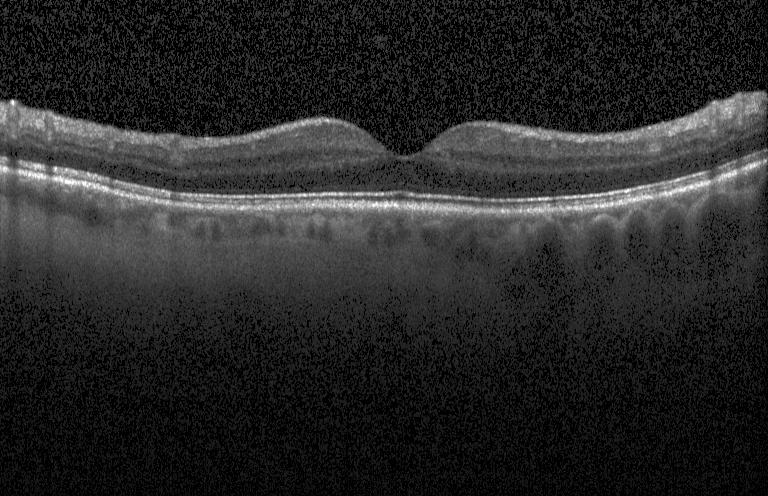
Spectral-domain optical coherence tomography · retinal OCT cross-section · horizontal scan through the fovea.
OCT finding: no evidence of CNV, DME, or drusen.